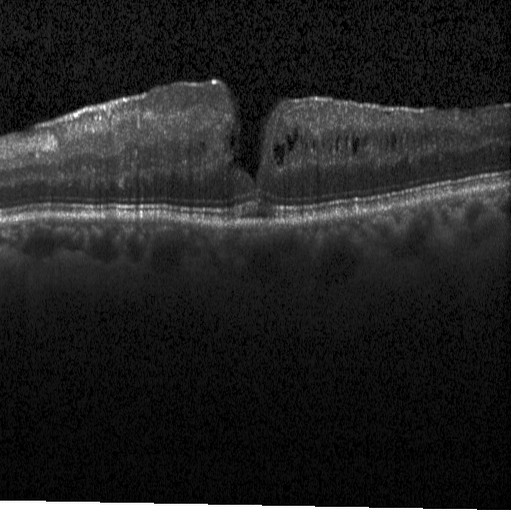
Diagnosis: DME.